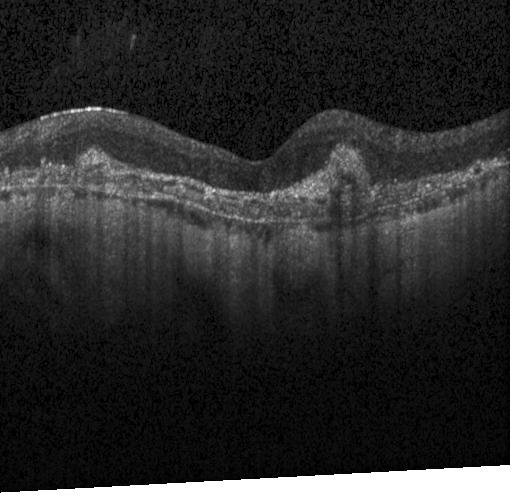 The scan shows choroidal neovascularization.